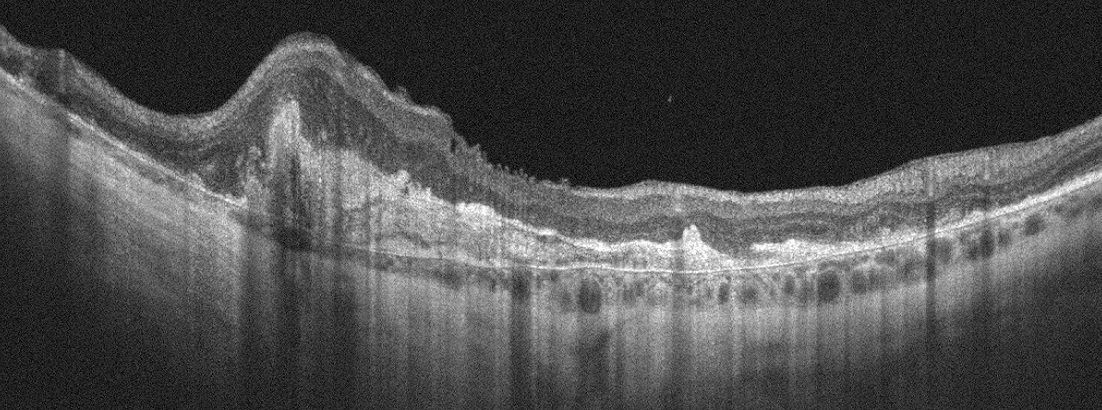

Optical coherence tomography scan, through the macula. Diagnosis: age-related macular degeneration (AMD).